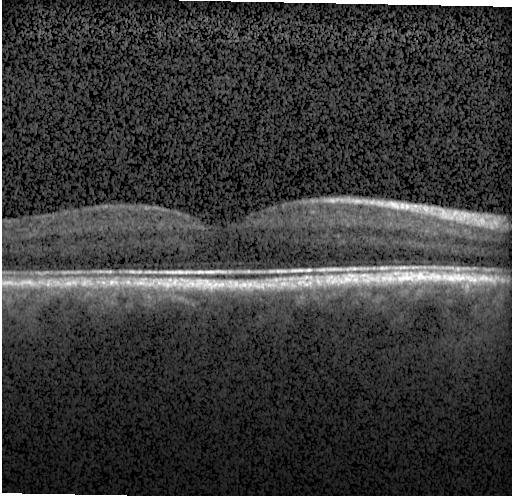
Diagnosis: no choroidal neovascularization, diabetic macular edema, or drusen.